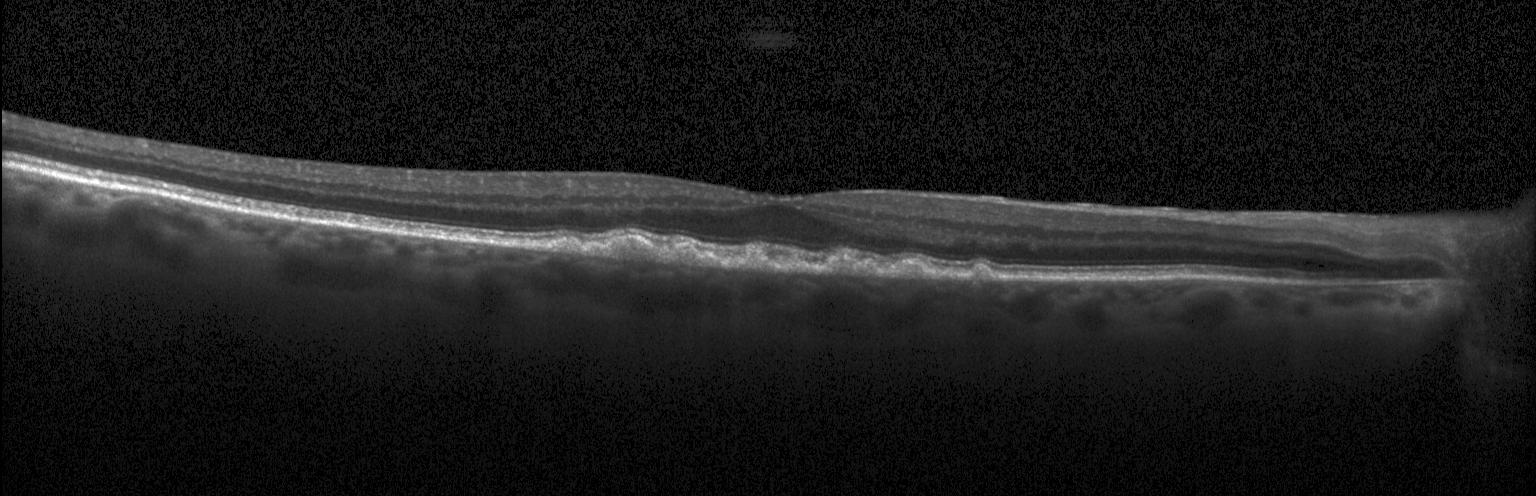
Optical coherence tomography scan.
This B-scan demonstrates sub-RPE drusenoid deposits.